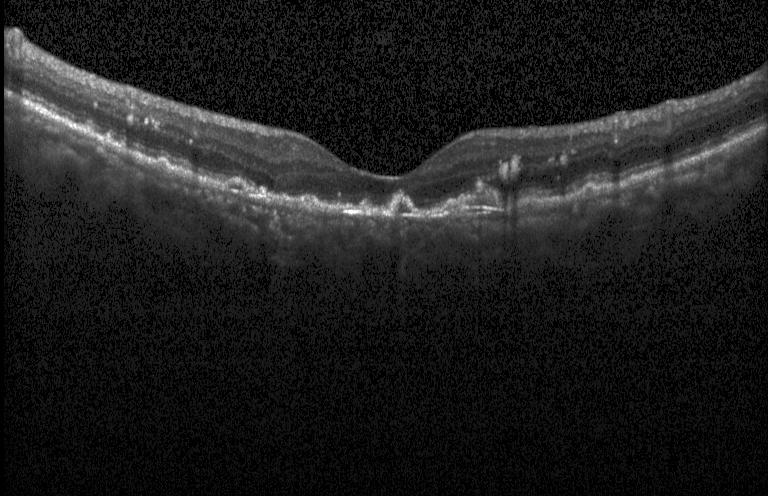
Finding: choroidal neovascularization (CNV).